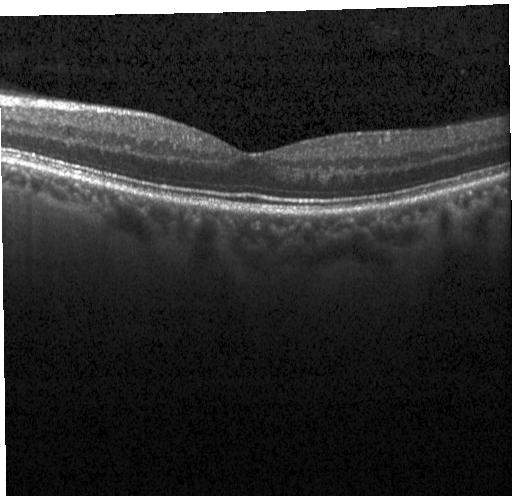
Impression: no evidence of CNV, DME, or drusen.